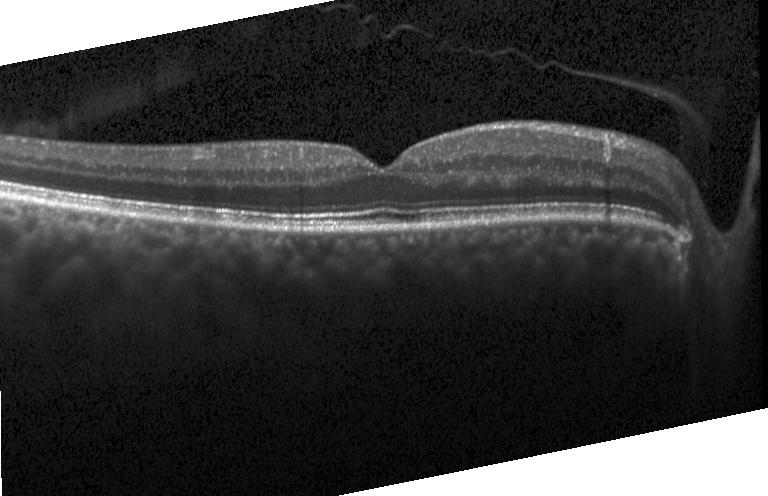
OCT B-scan
Diagnosis: neither choroidal neovascularization, diabetic macular edema, nor drusen.